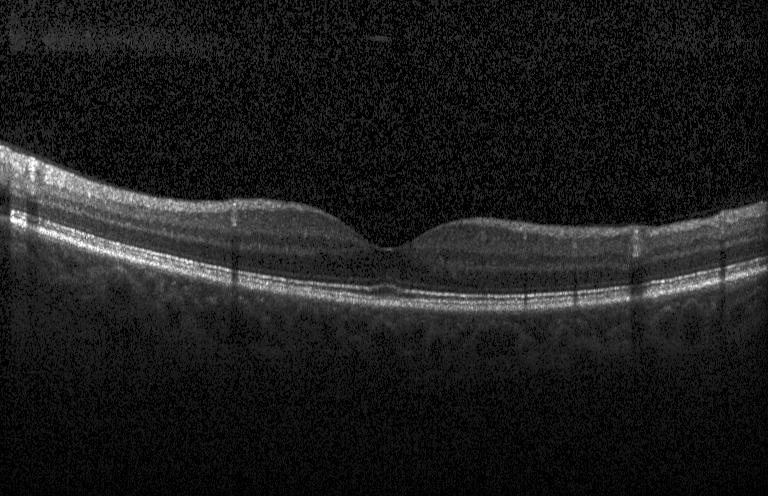
Retinal OCT B-scan — Diagnosis: neither CNV, DME, nor drusen.